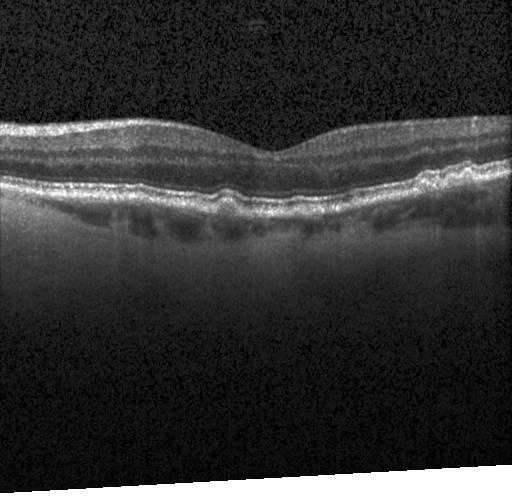 Centered on the fovea. Retinal OCT cross-section. Heidelberg Spectralis OCT system. Finding: drusen.